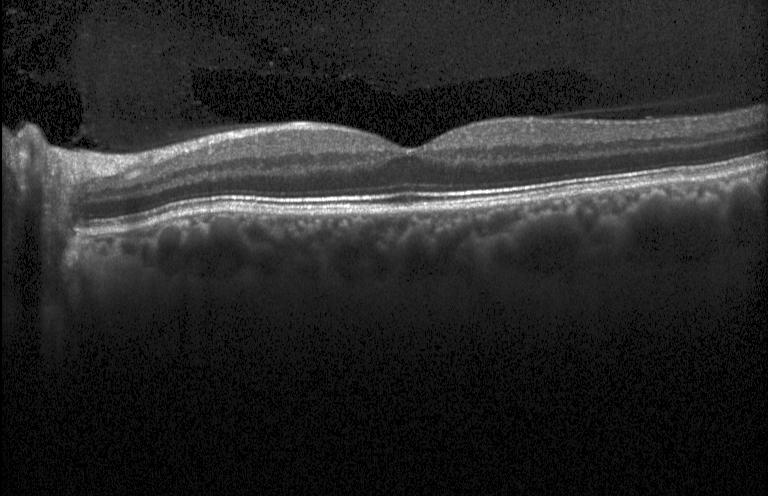

Spectral-domain OCT · OCT line scan. OCT finding: no choroidal neovascularization, diabetic macular edema, or drusen.